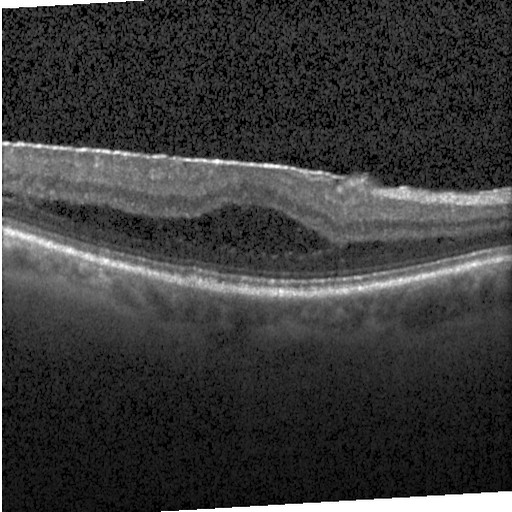

Optical coherence tomography scan. SD-OCT. Heidelberg Spectralis. The scan shows diabetic macular edema (DME).